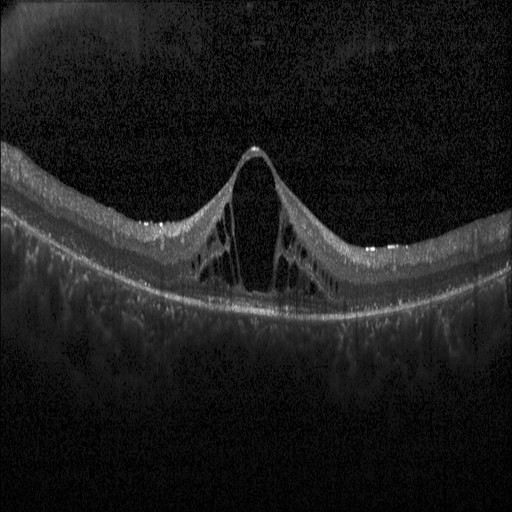

Heidelberg Spectralis; spectral-domain OCT; retinal OCT cross-section
DME.